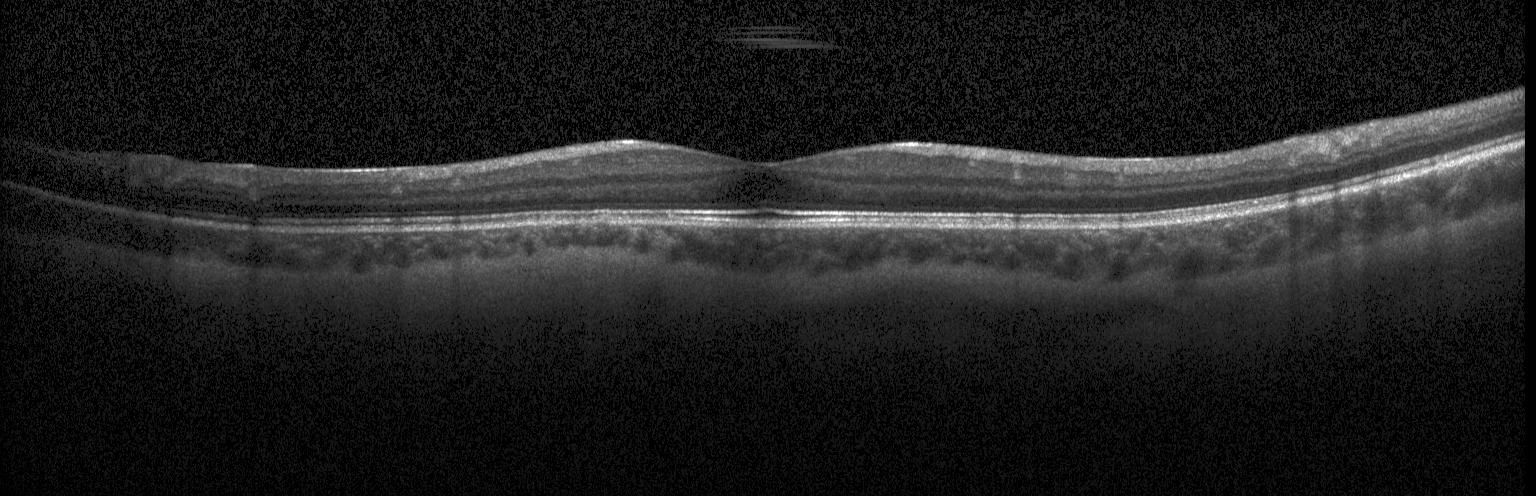

No evidence of choroidal neovascularization, diabetic macular edema, or drusen.